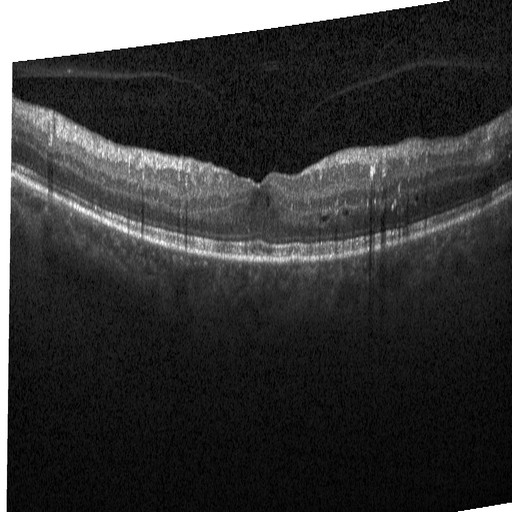

Finding: diabetic macular edema.